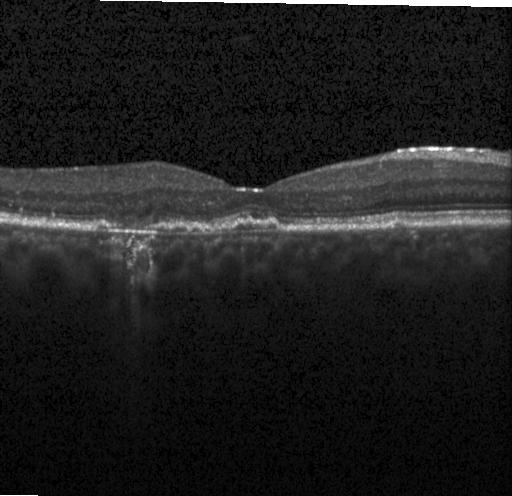
Horizontal scan through the fovea, optical coherence tomography B-scan. Diagnosis: choroidal neovascularization.